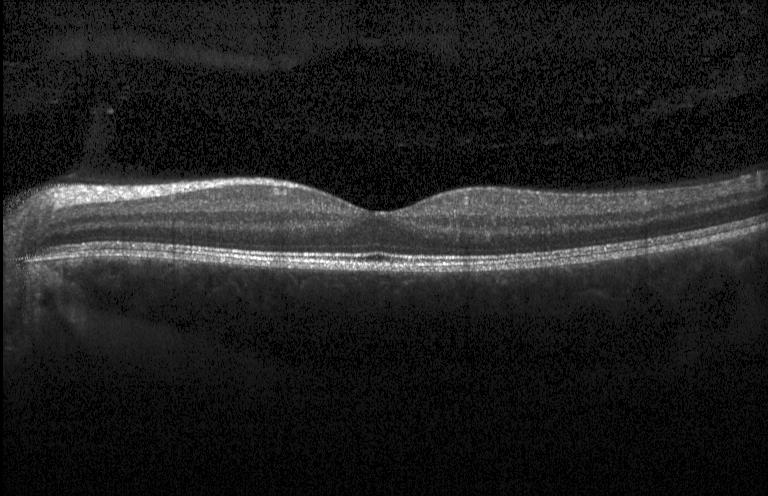
Dx: neither CNV, DME, nor drusen.